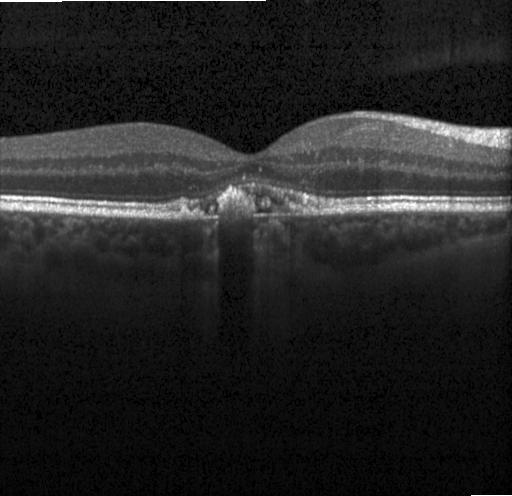 The scan shows choroidal neovascularization.